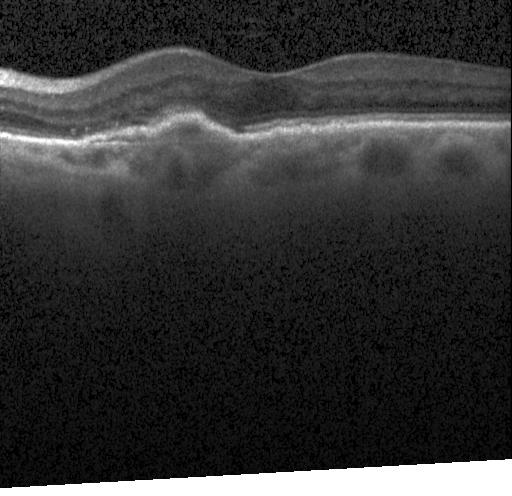
Acquired on a Heidelberg Spectralis. Fovea-centered. OCT B-scan. Spectral-domain OCT. Macular OCT: a choroidal neovascular membrane.